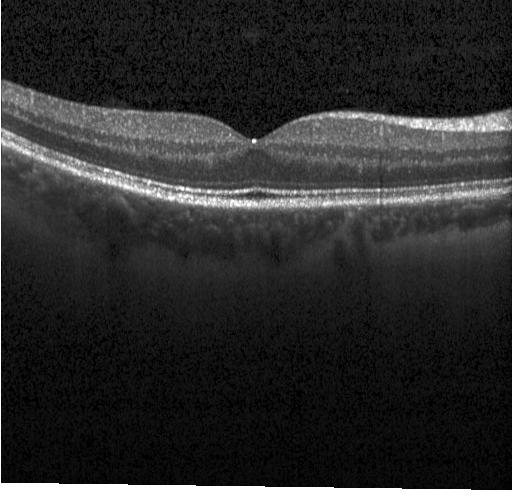

Neither CNV, DME, nor drusen.